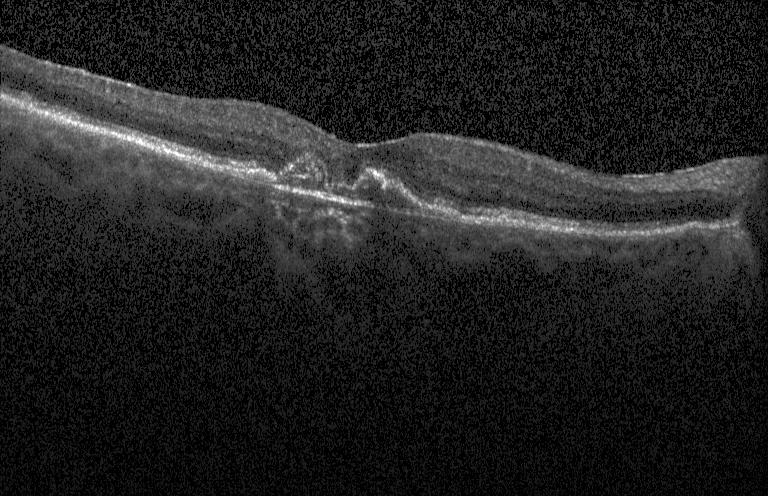
Macular OCT demonstrating a choroidal neovascular membrane.